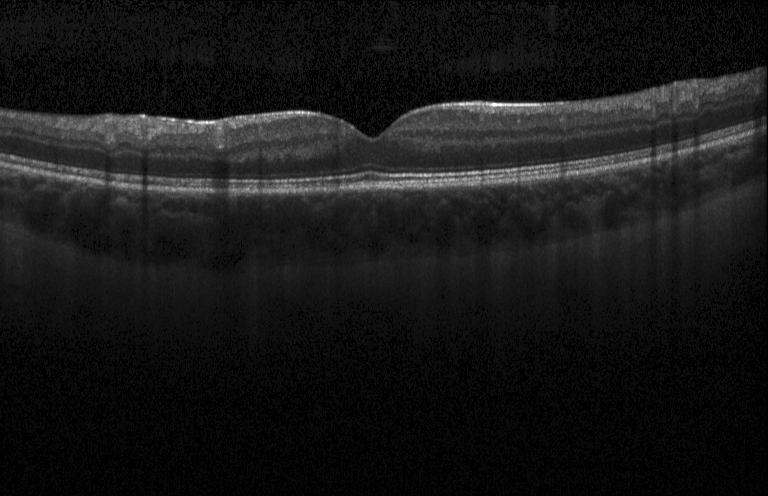

Retinal OCT cross-section. Finding: no evidence of choroidal neovascularization, diabetic macular edema, or drusen.